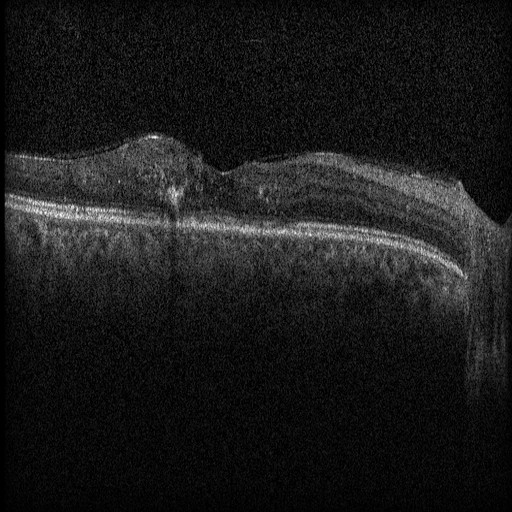

Impression: diabetic macular edema (DME).